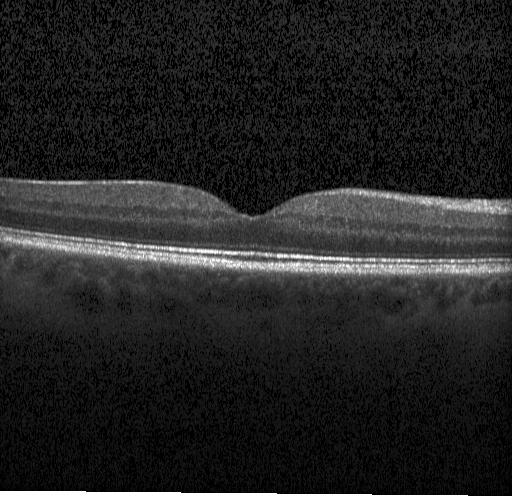
OCT scan showing no CNV, no DME, and no drusen.